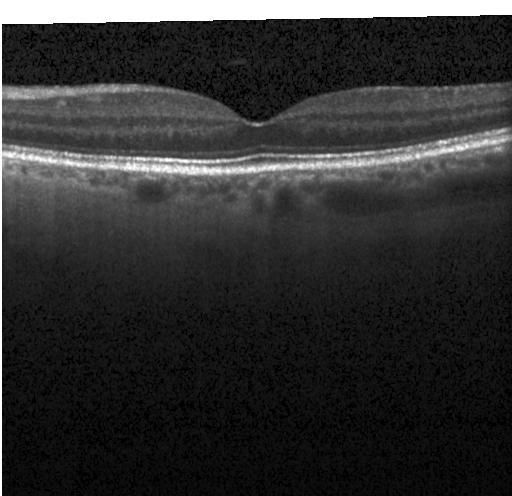

Acquired on a Heidelberg Spectralis; OCT line scan; centered on the fovea.
Finding: no CNV, DME, or drusen.